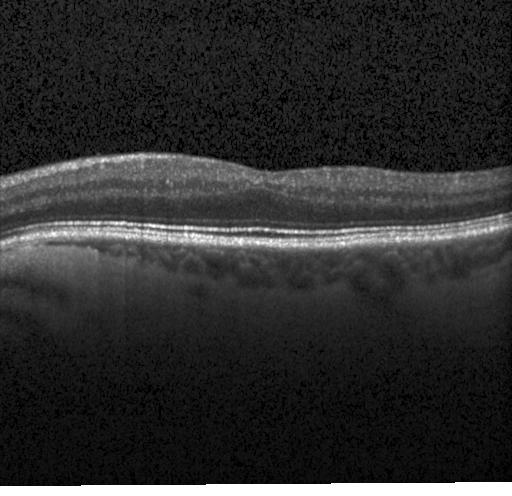

This B-scan demonstrates no evidence of CNV, DME, or drusen.